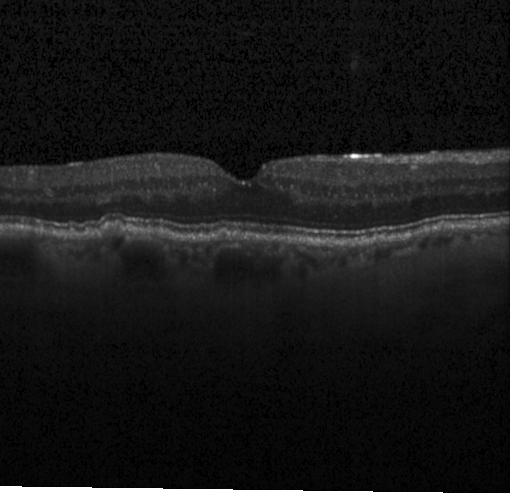

Retinal OCT cross-section
Assessment: drusen.